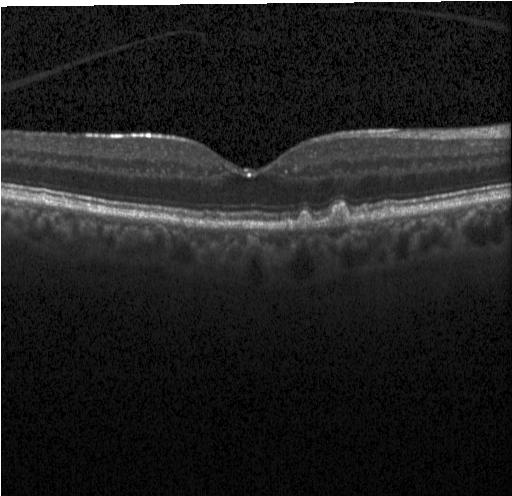 Macular scan · SD-OCT · Heidelberg Spectralis · retinal OCT B-scan. Diagnosis: multiple drusen.